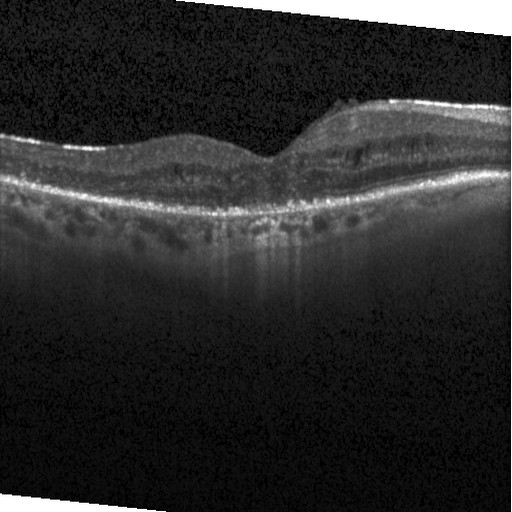
Macular OCT: DME.